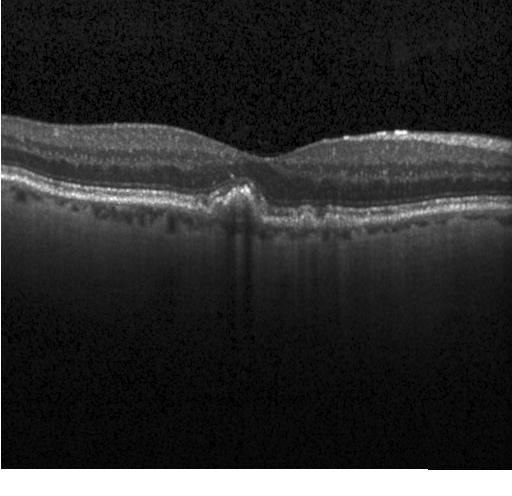

Macular OCT: sub-RPE drusenoid deposits.